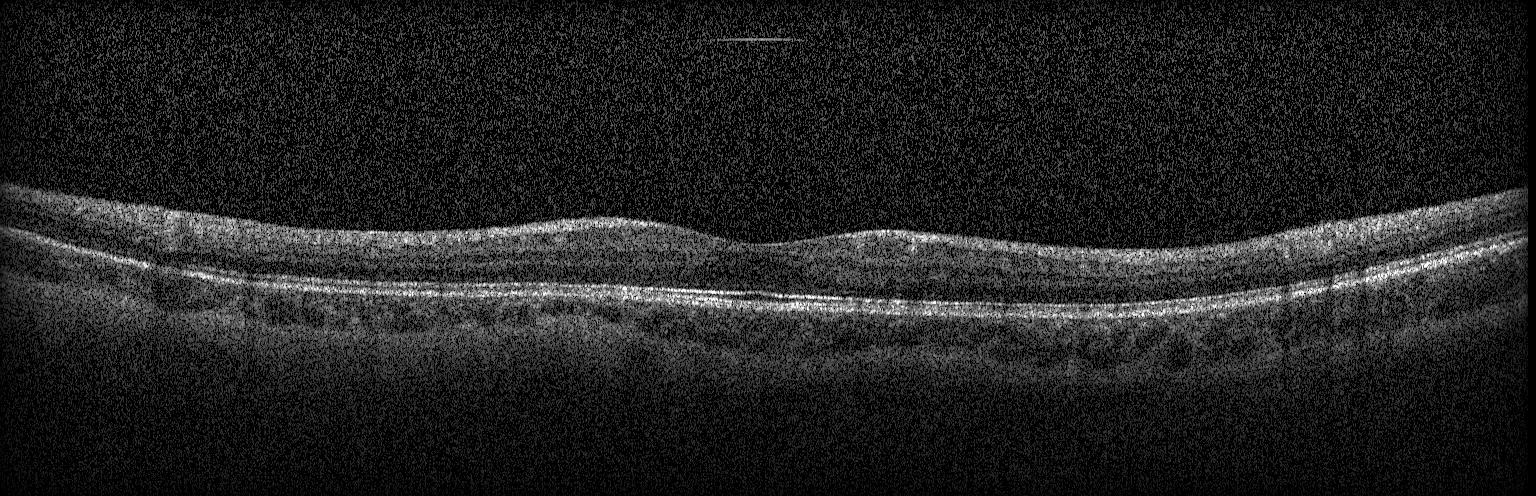

Spectral-domain OCT · acquired on a Heidelberg Spectralis · macular scan · OCT B-scan. Impression: neither choroidal neovascularization, diabetic macular edema, nor drusen.